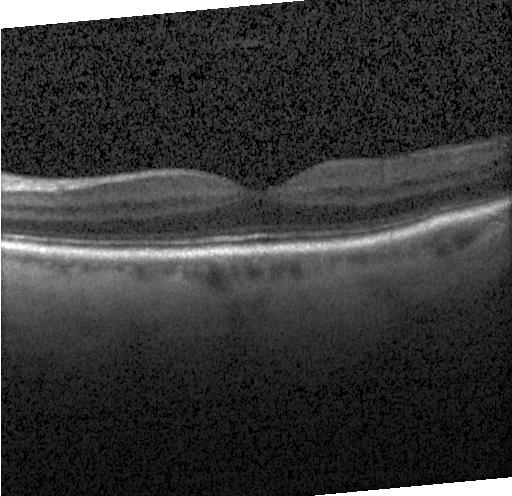 SD-OCT; OCT line scan; Heidelberg Spectralis OCT system. This B-scan demonstrates no choroidal neovascularization, no diabetic macular edema, and no drusen.